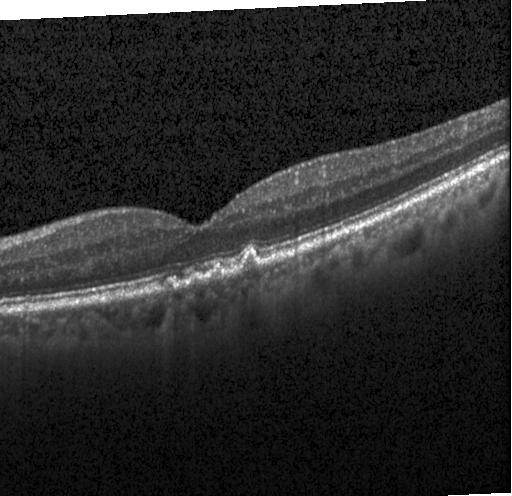 OCT line scan
The scan shows multiple drusen.